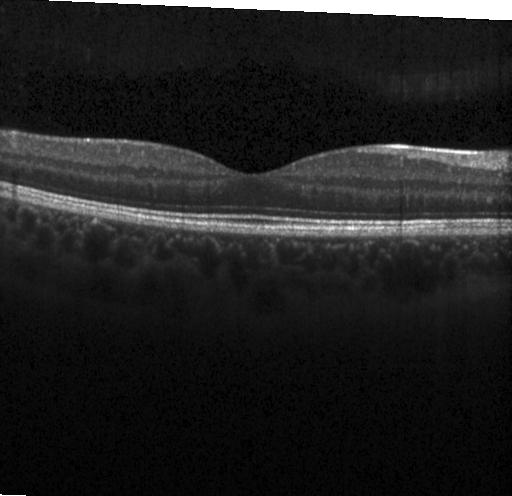
OCT line scan
Diagnosis: no choroidal neovascularization, no diabetic macular edema, and no drusen.